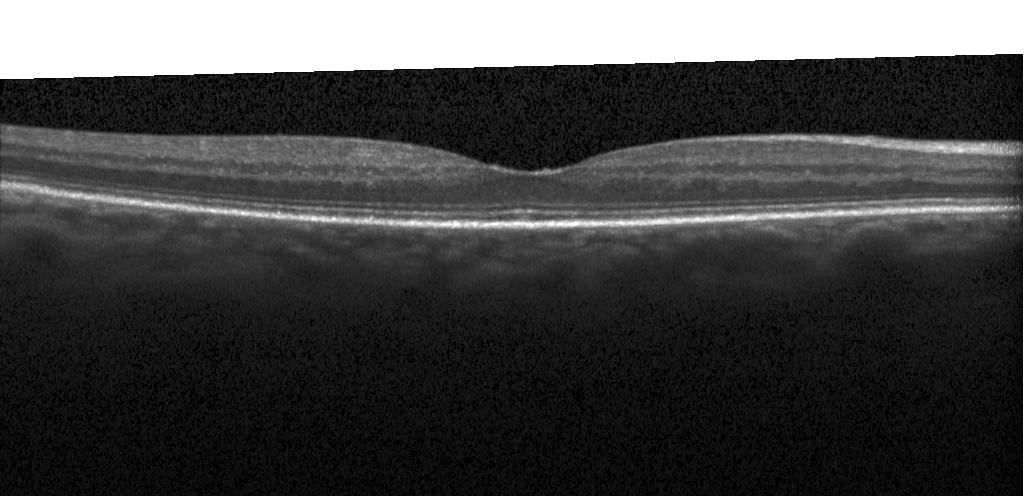
Impression: no CNV, DME, or drusen.